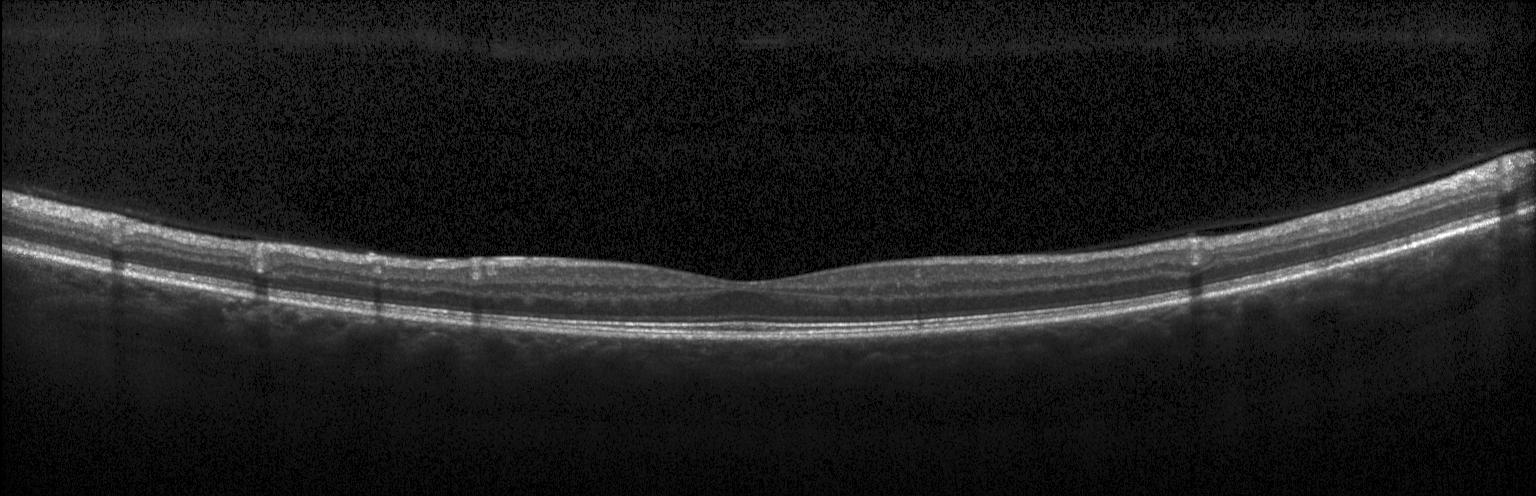
Retinal OCT B-scan.
The scan shows no choroidal neovascularization, diabetic macular edema, or drusen.